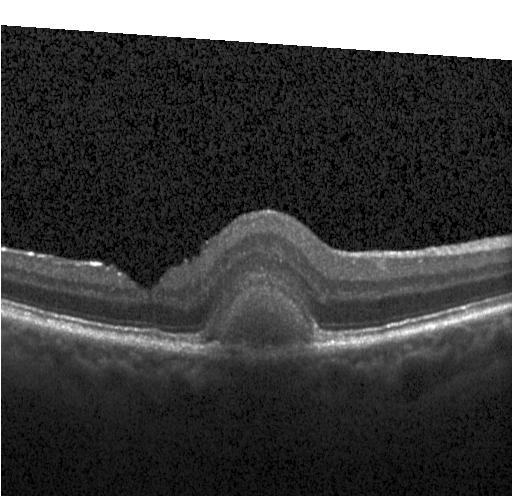
Impression: a choroidal neovascular membrane.